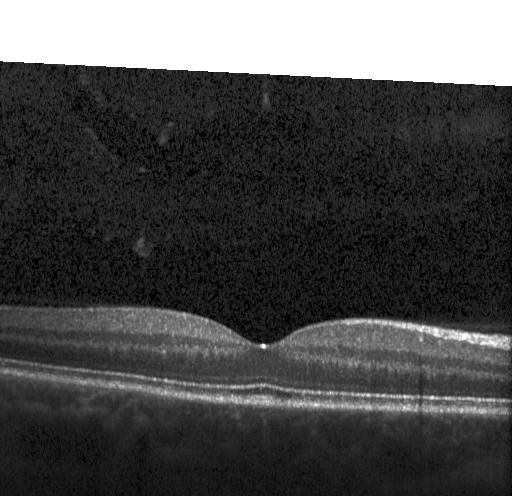

Macular OCT: neither choroidal neovascularization, diabetic macular edema, nor drusen.